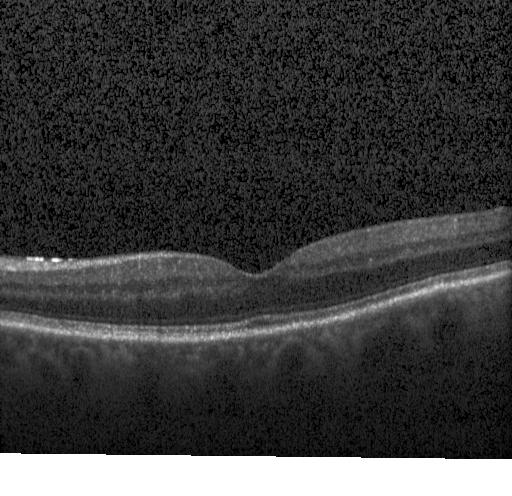 Macular OCT: no evidence of choroidal neovascularization, diabetic macular edema, or drusen.